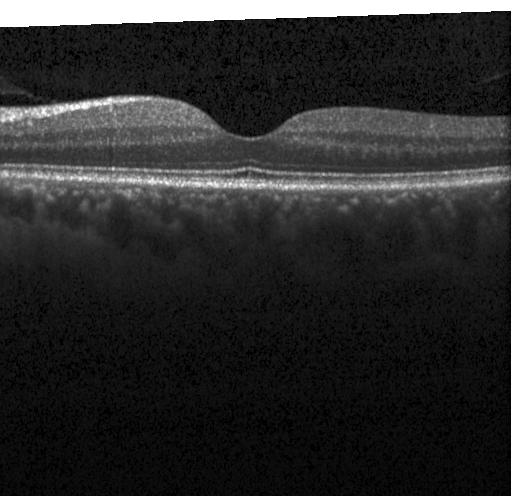
Dx: neither CNV, DME, nor drusen.